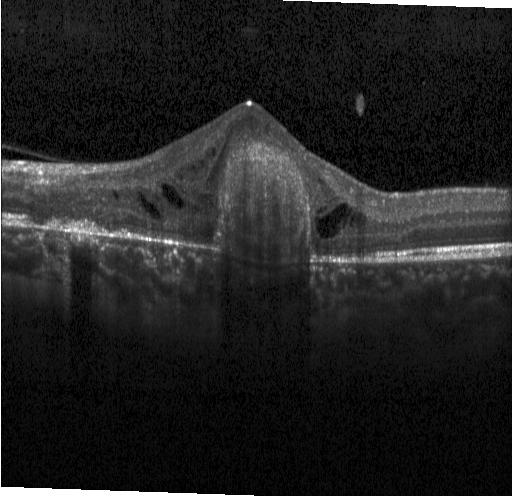

Centered on the fovea · OCT line scan · instrument: Heidelberg Spectralis — Finding: a choroidal neovascular membrane.